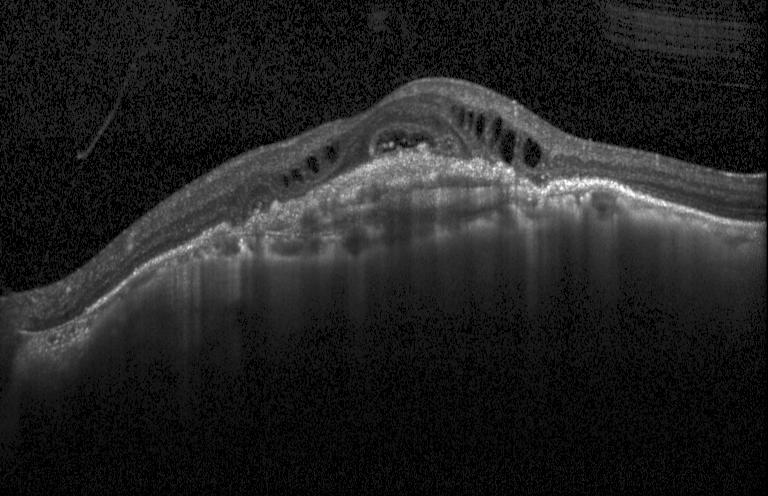

OCT scan showing a choroidal neovascular membrane.